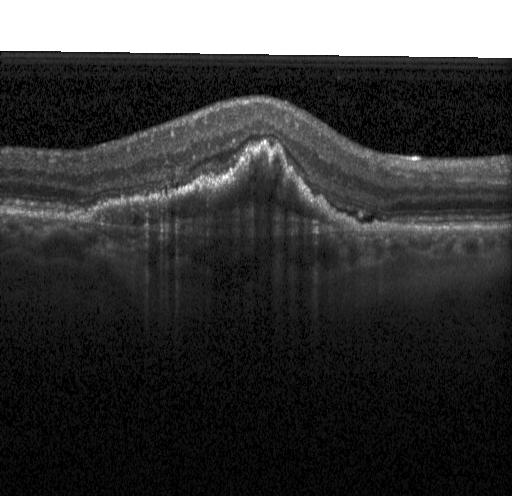
Spectral-domain optical coherence tomography; OCT line scan.
A choroidal neovascular membrane.